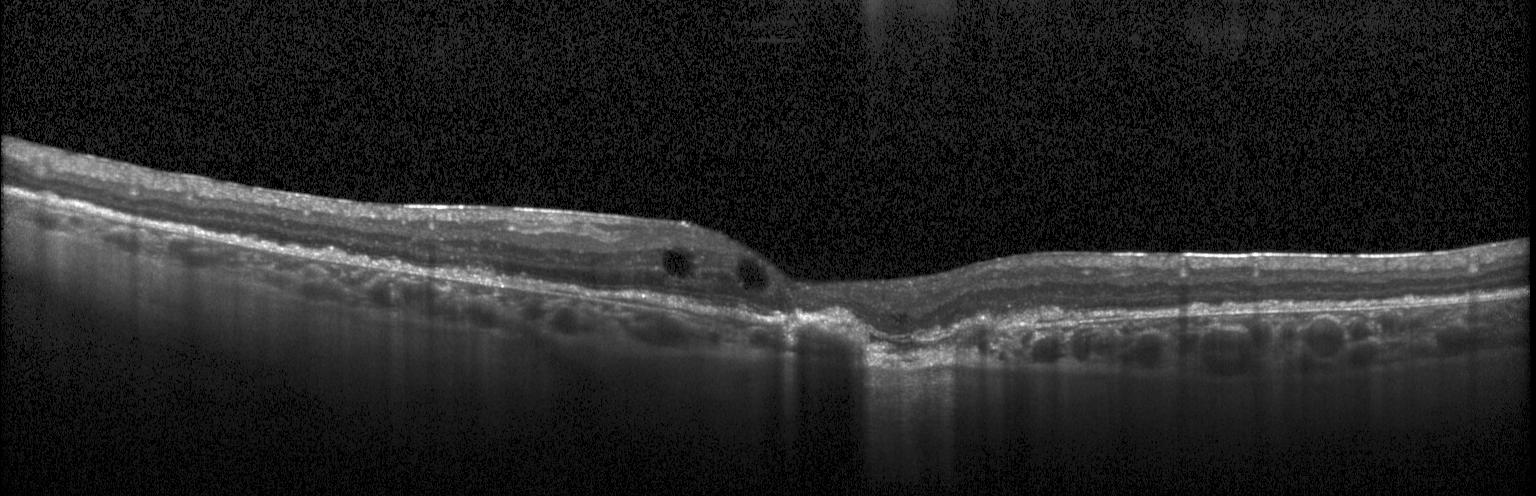

Finding: a choroidal neovascular membrane.